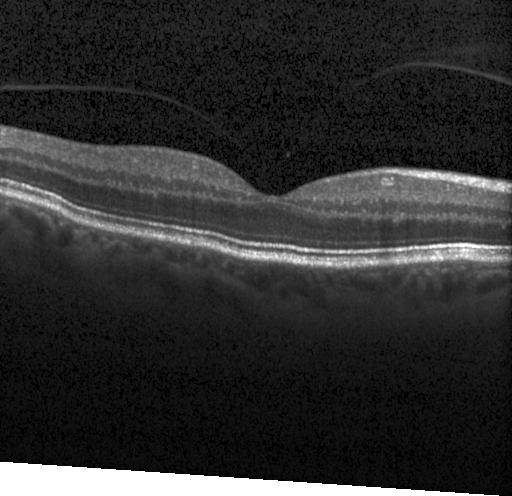 Optical coherence tomography B-scan.
Assessment: no CNV, no DME, and no drusen.